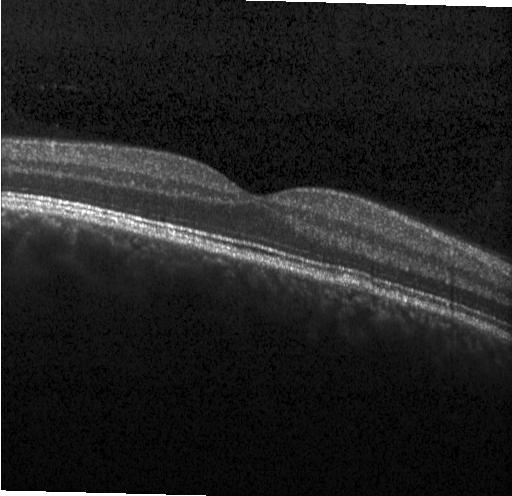 SD-OCT; Heidelberg Spectralis; retinal OCT B-scan; through the macula.
Diagnosis: no choroidal neovascularization, diabetic macular edema, or drusen.